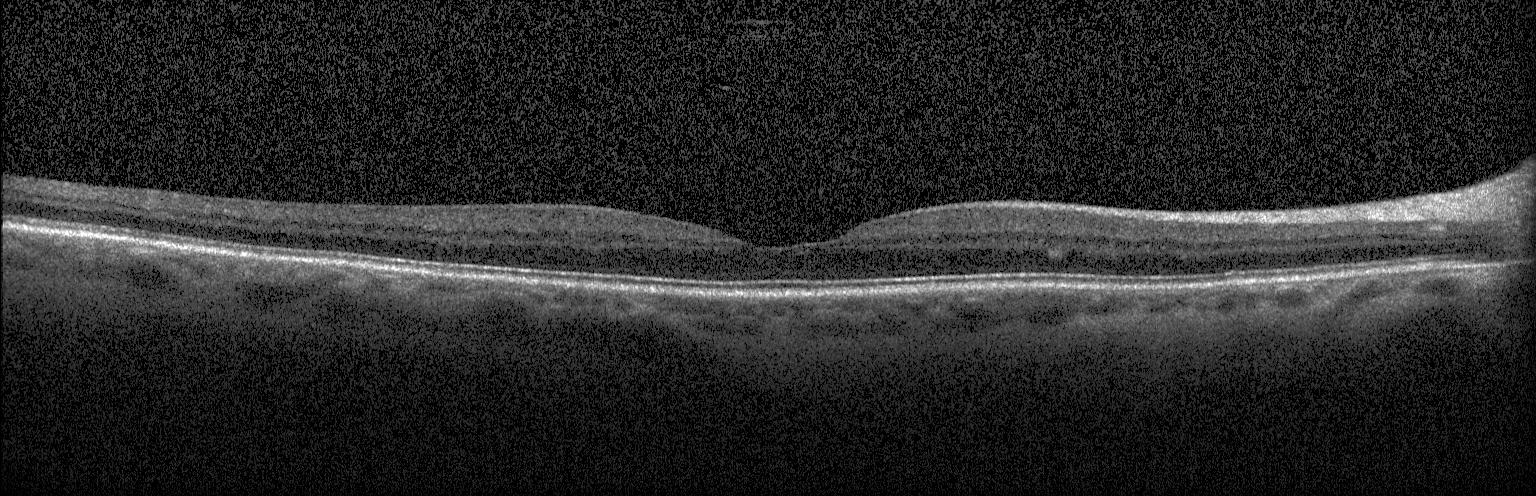

The scan shows neither choroidal neovascularization, diabetic macular edema, nor drusen.